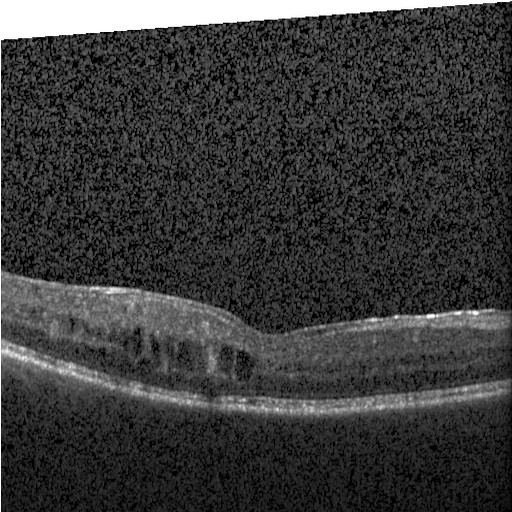
Macular OCT: diabetic macular edema.